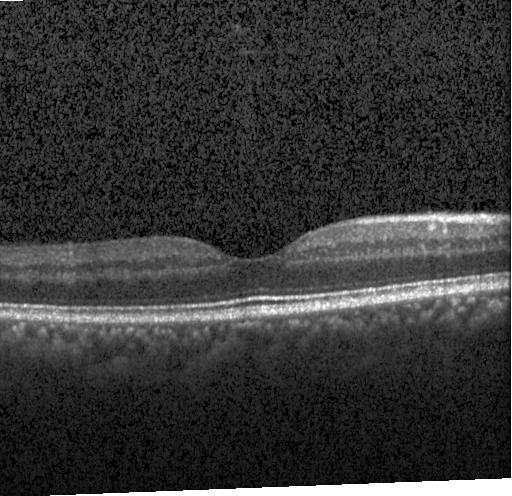
Finding: neither CNV, DME, nor drusen.